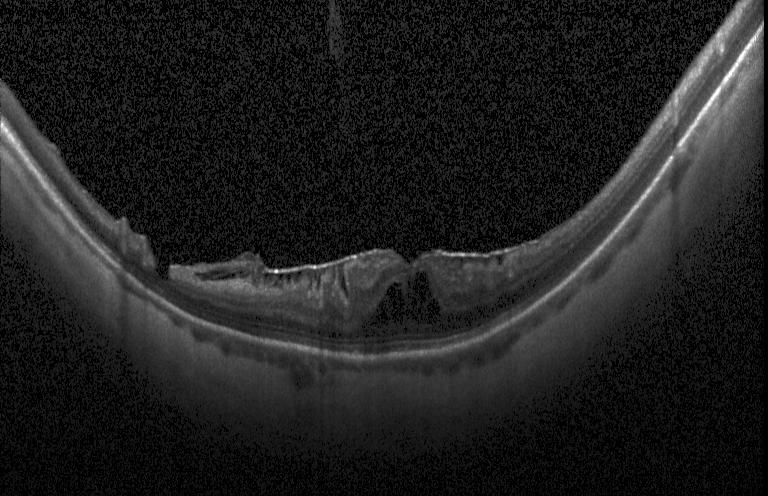

Heidelberg Spectralis OCT system · horizontal scan through the fovea · optical coherence tomography scan. DME.